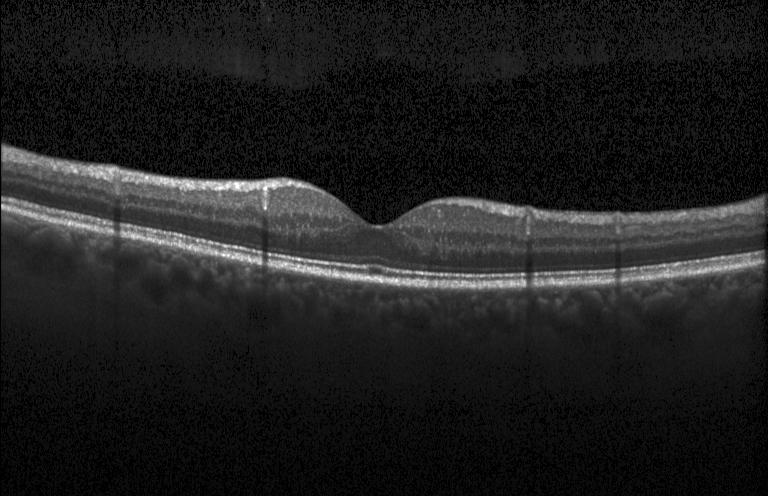 Dx: no CNV, DME, or drusen.